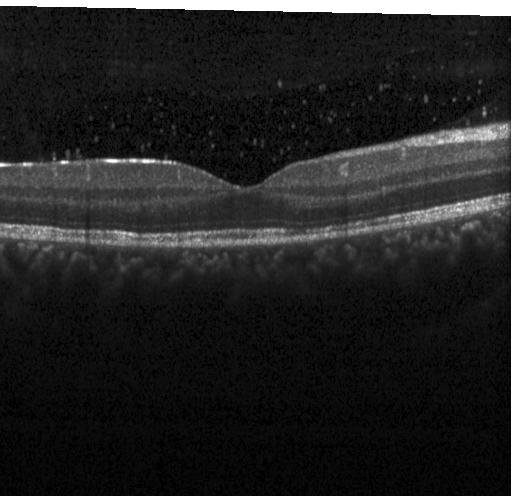

Retinal OCT B-scan. This B-scan demonstrates no choroidal neovascularization, no diabetic macular edema, and no drusen.